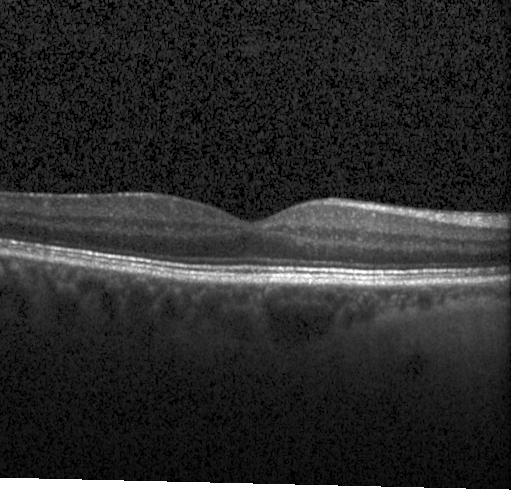
Finding: no evidence of choroidal neovascularization, diabetic macular edema, or drusen.